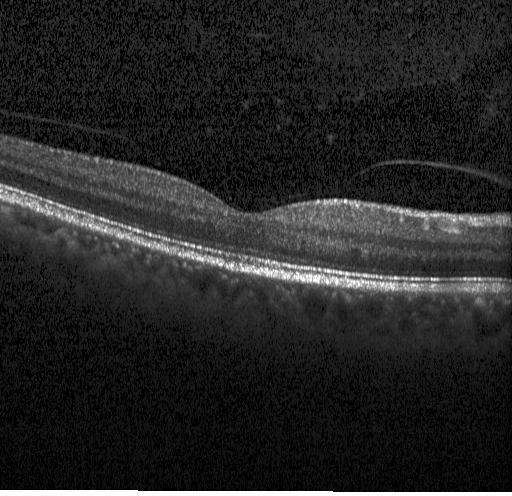

Horizontal scan through the fovea. Retinal OCT B-scan. Instrument: Heidelberg Spectralis
No choroidal neovascularization, diabetic macular edema, or drusen.